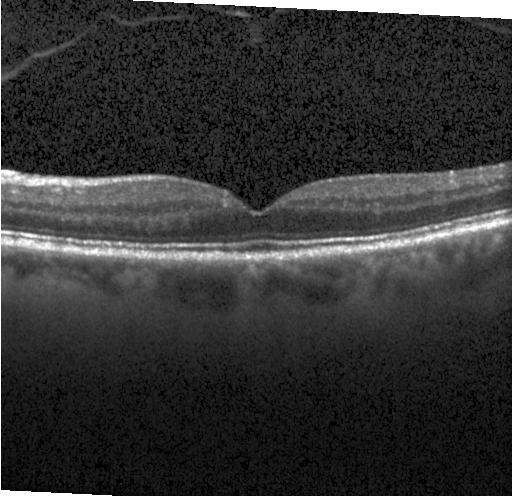 Diagnosis: no choroidal neovascularization, diabetic macular edema, or drusen.